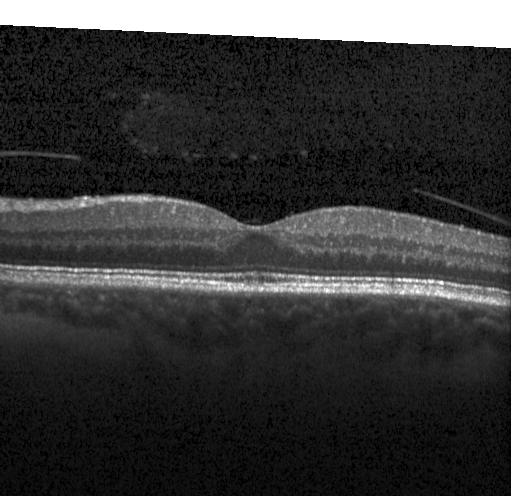 OCT B-scan showing no choroidal neovascularization, diabetic macular edema, or drusen.